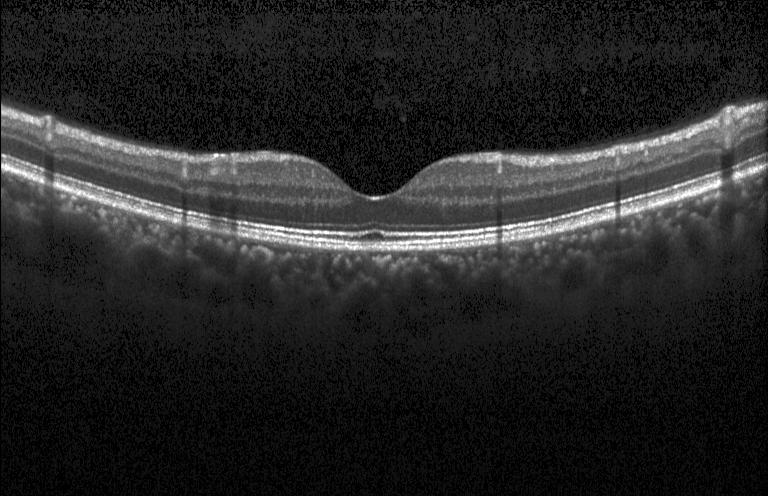 Retinal OCT cross-section · horizontal scan through the fovea. Diagnosis: no CNV, DME, or drusen.